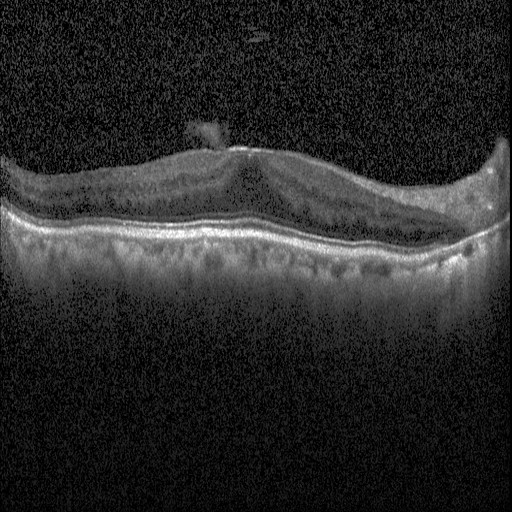
DME.